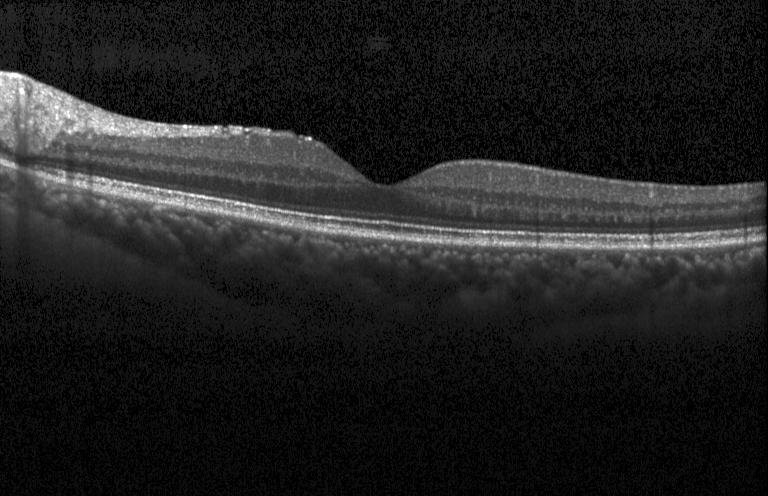
This B-scan demonstrates no choroidal neovascularization, no diabetic macular edema, and no drusen.